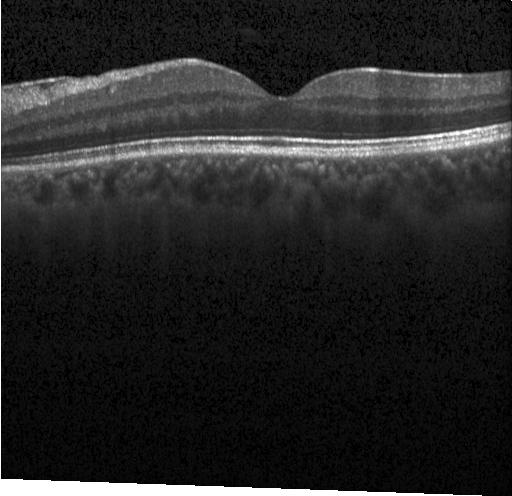
Impression: neither choroidal neovascularization, diabetic macular edema, nor drusen.